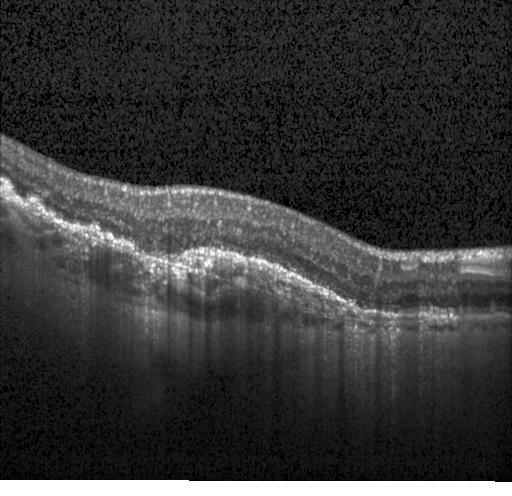
Finding: choroidal neovascularization.